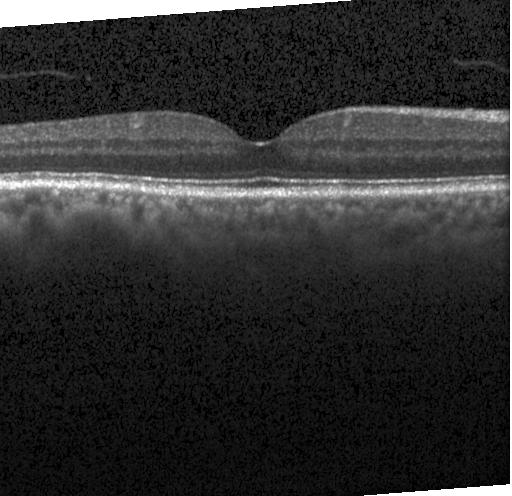 OCT line scan. Impression: no choroidal neovascularization, diabetic macular edema, or drusen.